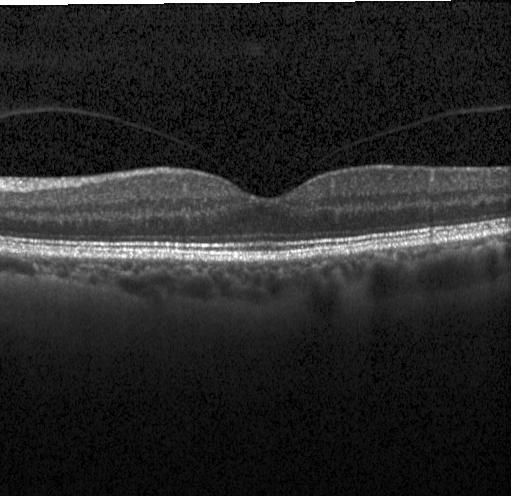 OCT line scan — Impression: no choroidal neovascularization, no diabetic macular edema, and no drusen.